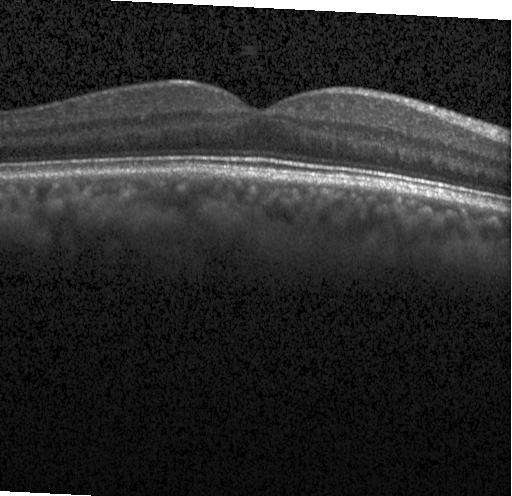

Through the macula. SD-OCT. OCT line scan. Acquired on a Heidelberg Spectralis
Finding: no choroidal neovascularization, no diabetic macular edema, and no drusen.